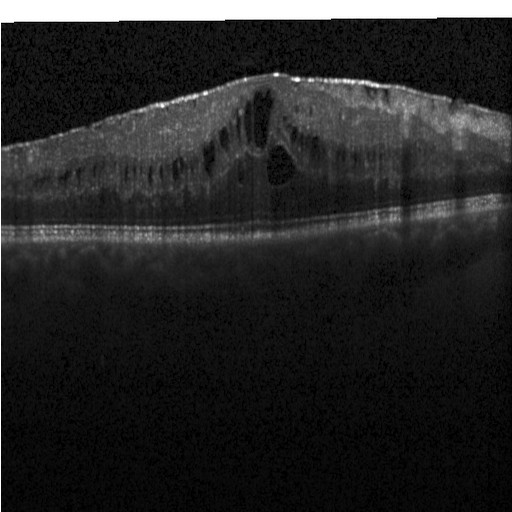

Heidelberg Spectralis; OCT line scan.
Impression: diabetic macular edema (DME).